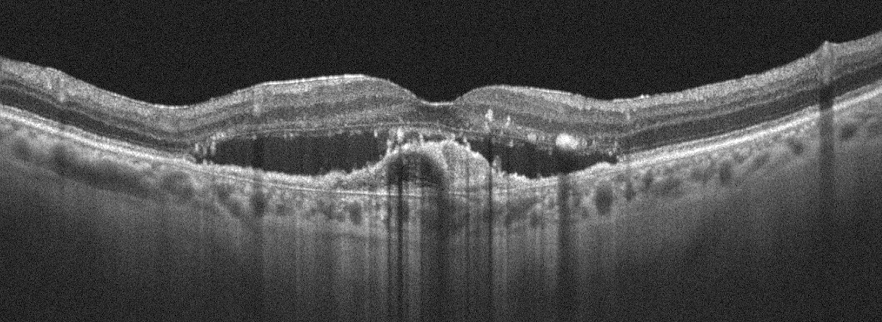 Acquired on an Optovue Avanti RTVue XR, left eye, through the macula, optical coherence tomography scan — Diagnosis: AMD.